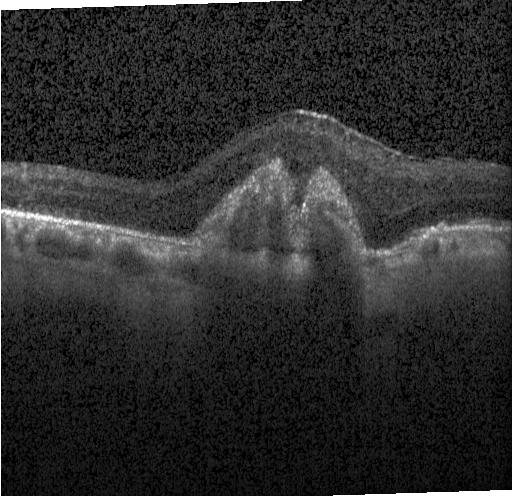

Dx: CNV.